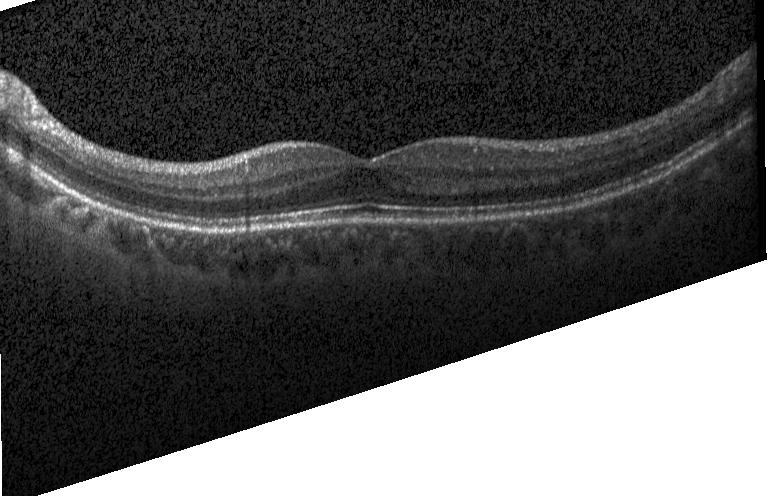 Fovea-centered, Heidelberg Spectralis, spectral-domain optical coherence tomography, retinal OCT cross-section.
Finding: no CNV, DME, or drusen.